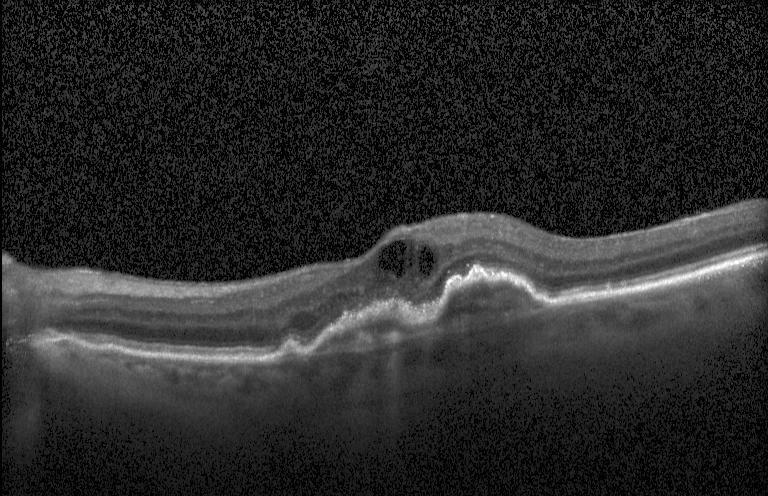 Spectral-domain OCT. Heidelberg Spectralis OCT system. OCT B-scan. Macular scan. Choroidal neovascularization (CNV).